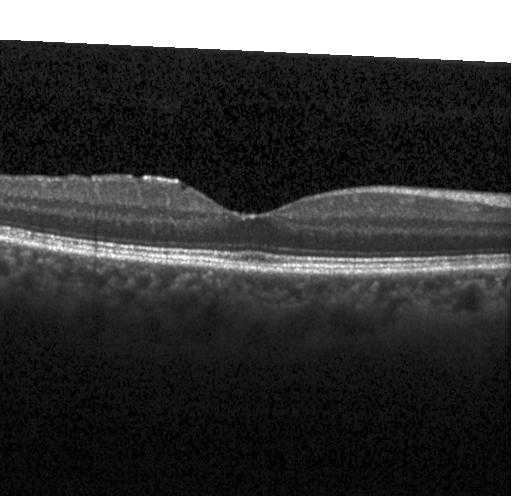
Retinal OCT B-scan; horizontal scan through the fovea; Heidelberg Spectralis OCT system. OCT finding: neither CNV, DME, nor drusen.